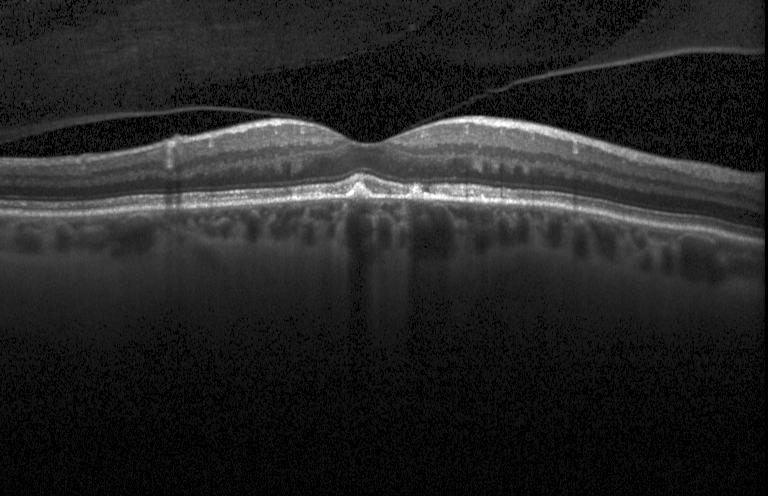

OCT B-scan, spectral-domain optical coherence tomography.
Finding: drusen.